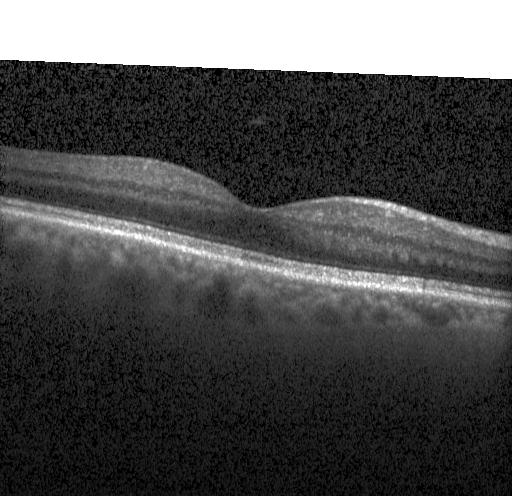

Finding: no choroidal neovascularization, no diabetic macular edema, and no drusen.